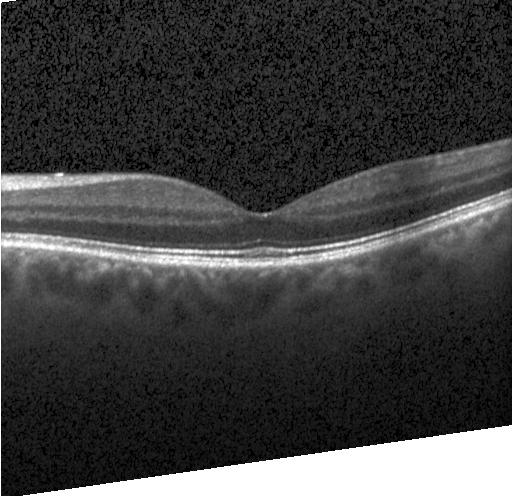

OCT B-scan. This B-scan demonstrates no choroidal neovascularization, no diabetic macular edema, and no drusen.